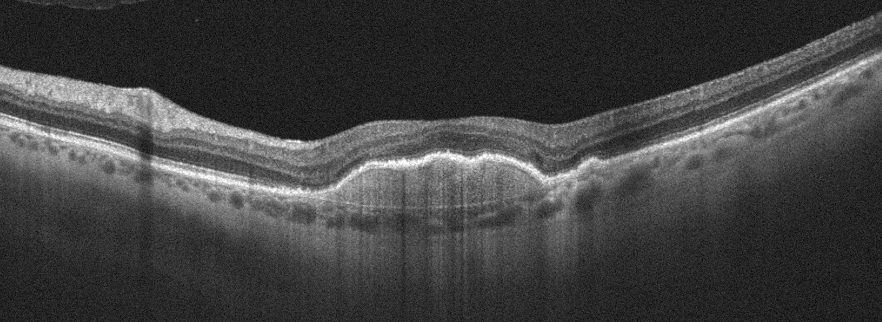

Retinal OCT B-scan; left eye — Impression: age-related macular degeneration (AMD).